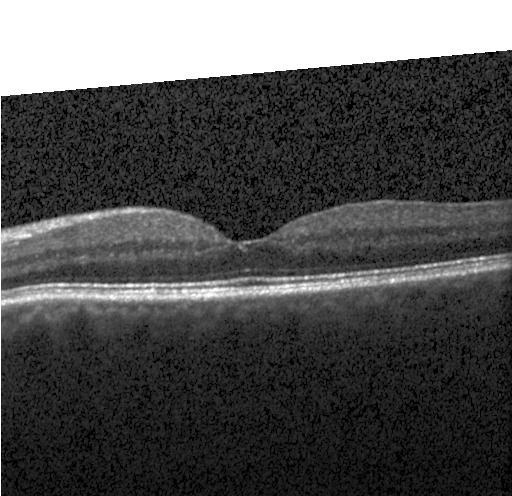

Retinal OCT B-scan
Impression: no evidence of choroidal neovascularization, diabetic macular edema, or drusen.